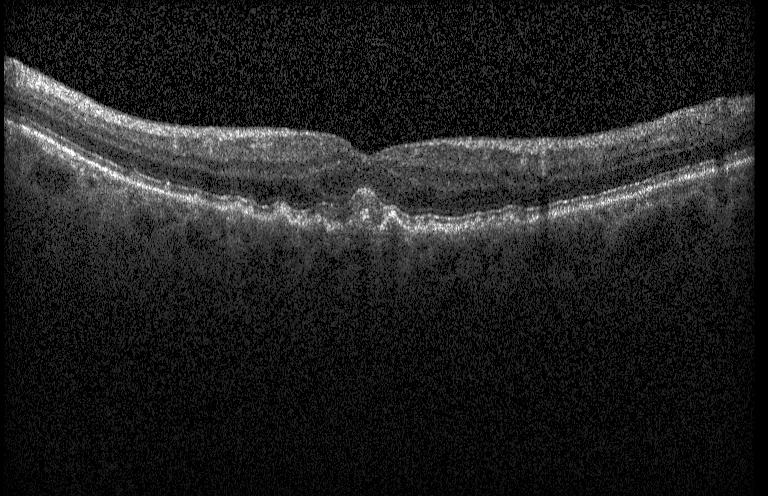 Heidelberg Spectralis OCT system; OCT line scan — Macular OCT: CNV.